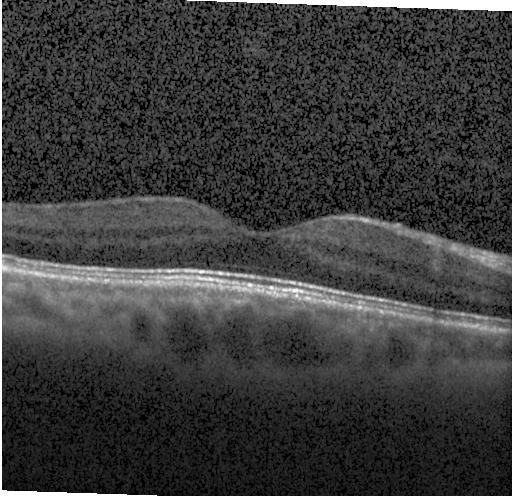
Optical coherence tomography scan · acquired on a Heidelberg Spectralis · spectral-domain OCT — Impression: neither CNV, DME, nor drusen.